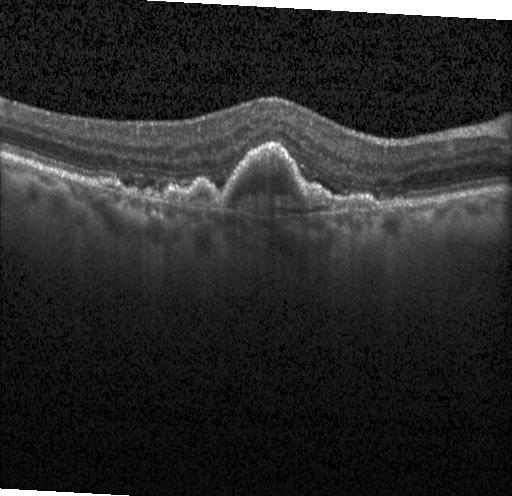

Retinal OCT B-scan. Finding: a choroidal neovascular membrane.